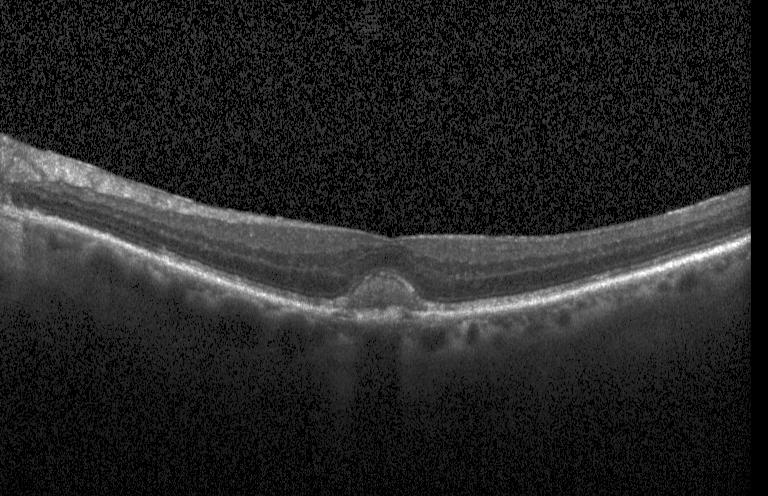
Retinal OCT B-scan
Macular OCT: CNV.